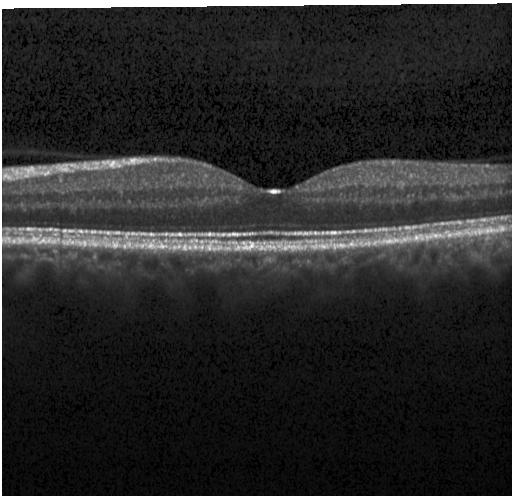
Spectral-domain optical coherence tomography; Heidelberg Spectralis; optical coherence tomography B-scan; centered on the fovea. OCT finding: no choroidal neovascularization, diabetic macular edema, or drusen.